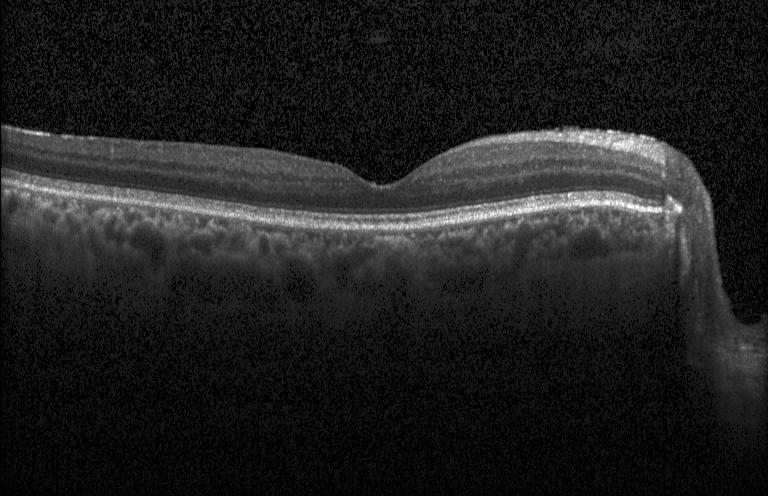 Retinal OCT B-scan · Heidelberg Spectralis OCT system · spectral-domain OCT · horizontal scan through the fovea — Finding: no choroidal neovascularization, diabetic macular edema, or drusen.